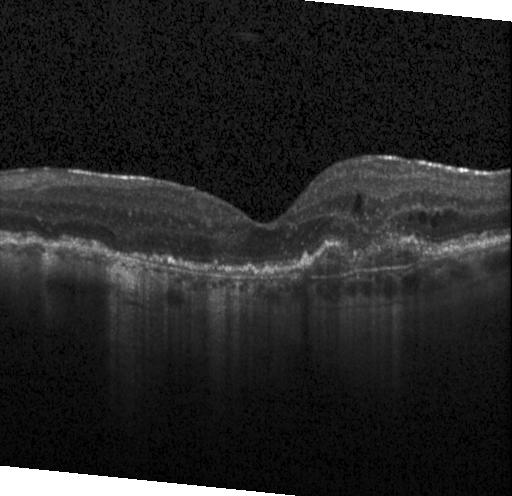

The scan shows a choroidal neovascular membrane.